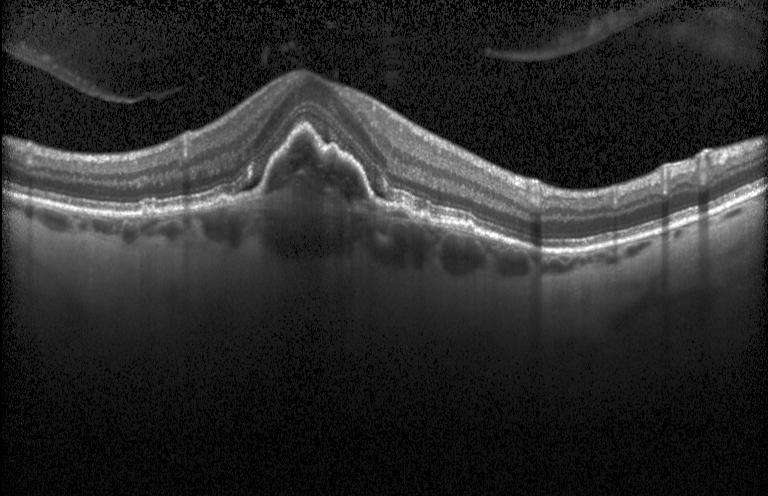

Optical coherence tomography scan · fovea-centered. OCT finding: a choroidal neovascular membrane.